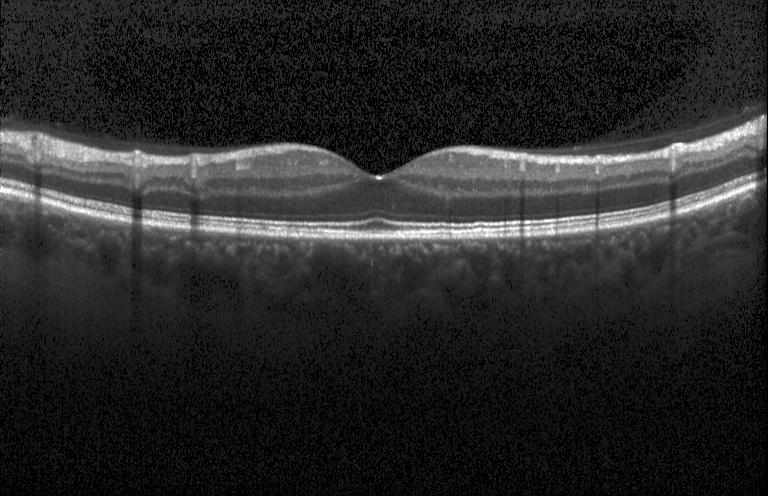
OCT B-scan showing neither choroidal neovascularization, diabetic macular edema, nor drusen.